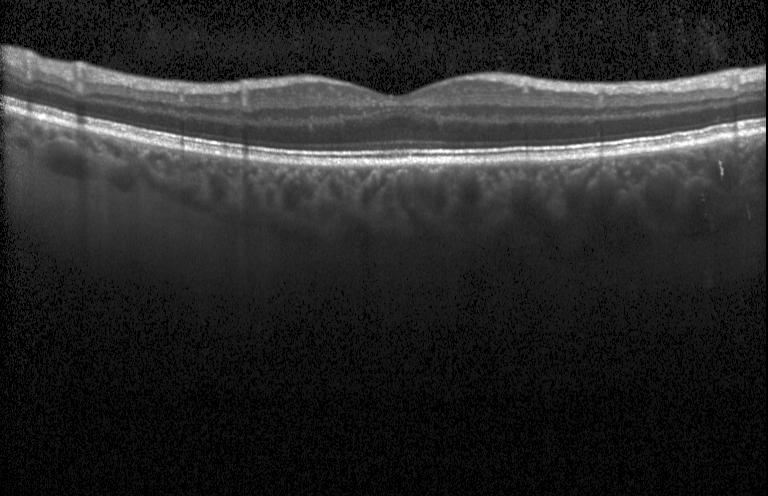

Acquired on a Heidelberg Spectralis; retinal OCT cross-section; fovea-centered
Finding: no evidence of choroidal neovascularization, diabetic macular edema, or drusen.